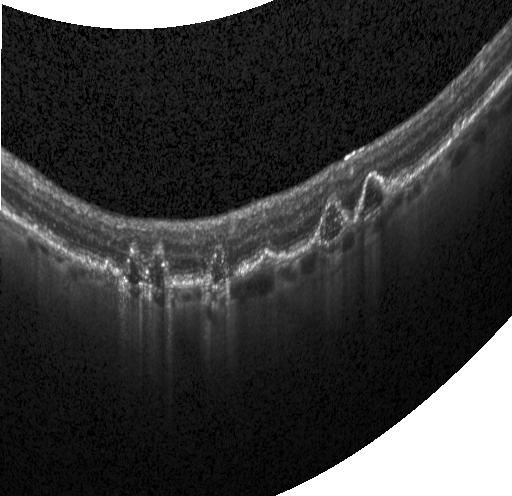

Retinal OCT cross-section; Heidelberg Spectralis OCT system; spectral-domain optical coherence tomography. Dx: a choroidal neovascular membrane.